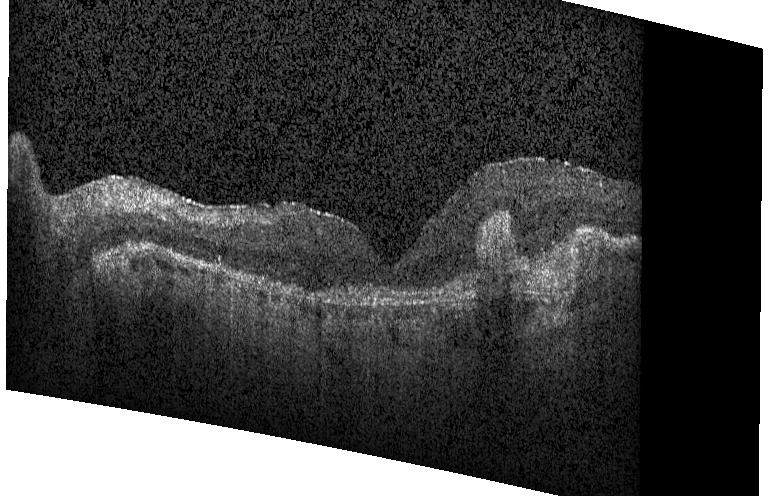
Assessment: a choroidal neovascular membrane.